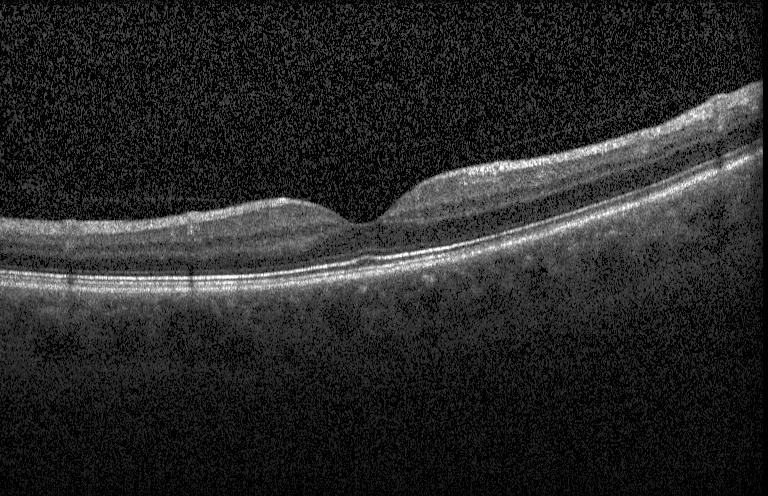

Finding: no choroidal neovascularization, diabetic macular edema, or drusen.